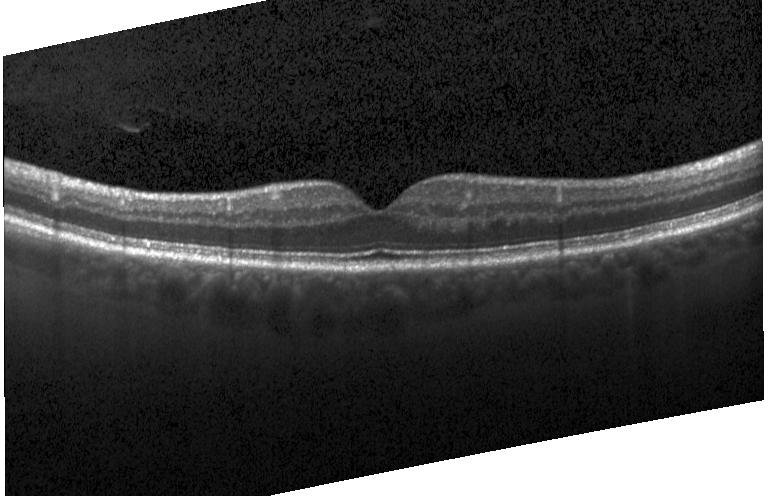 Optical coherence tomography scan.
Impression: no choroidal neovascularization, diabetic macular edema, or drusen.